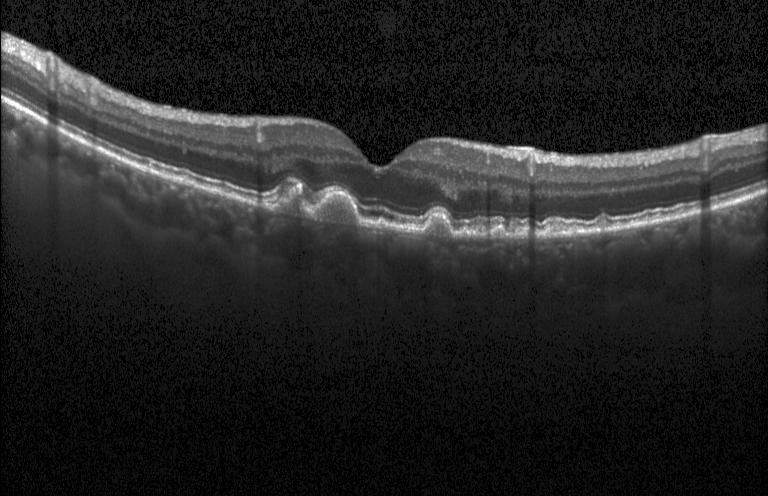

Optical coherence tomography B-scan — OCT finding: sub-RPE drusenoid deposits.